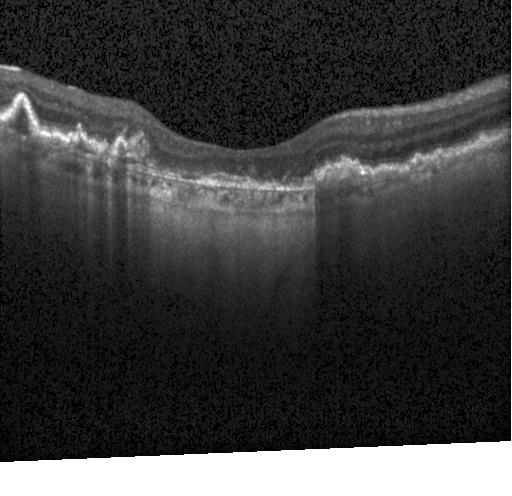

OCT line scan. Spectral-domain OCT. Through the macula.
Dx: choroidal neovascularization (CNV).